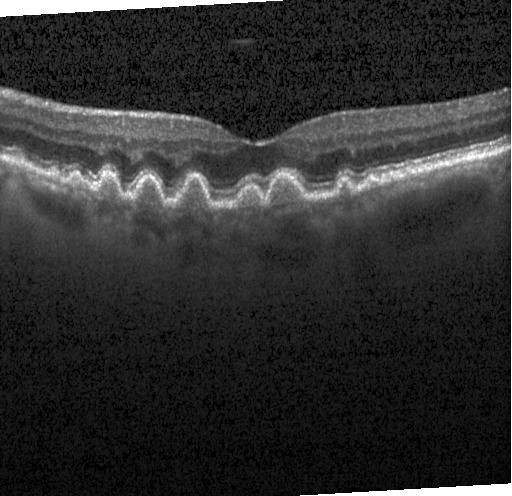 SD-OCT; optical coherence tomography scan
Impression: multiple drusen.